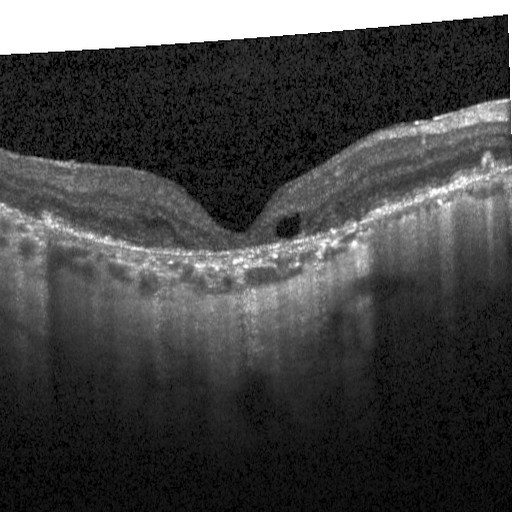
Retinal OCT cross-section
Diagnosis: diabetic macular edema.